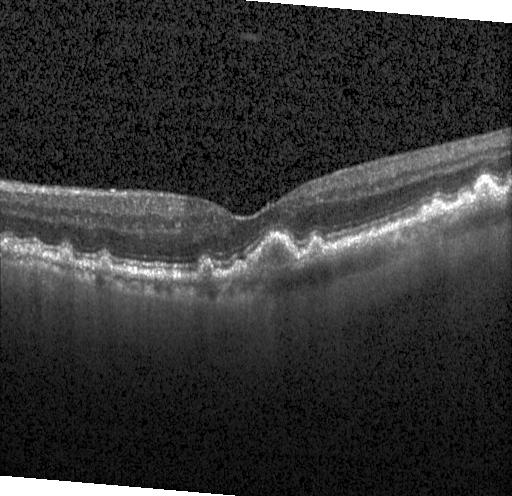

OCT B-scan
OCT finding: multiple drusen.